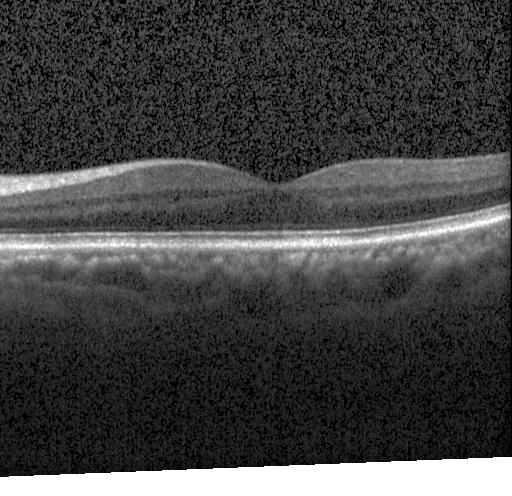

SD-OCT, OCT B-scan, acquired on a Heidelberg Spectralis — This B-scan demonstrates no CNV, no DME, and no drusen.